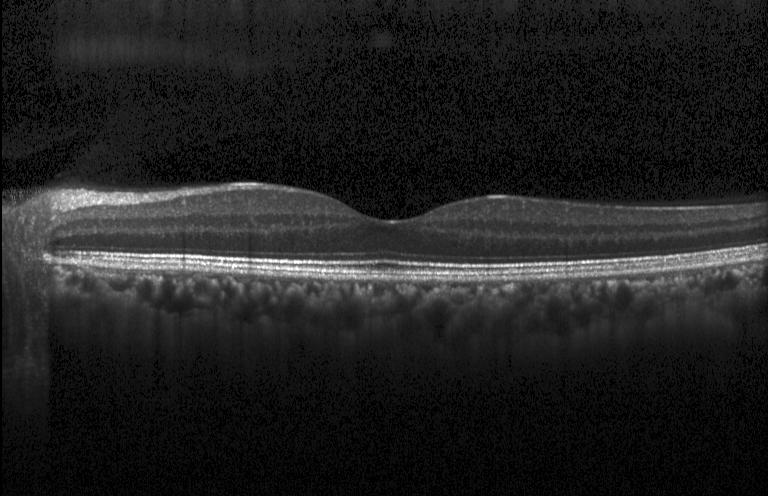

Centered on the fovea, spectral-domain optical coherence tomography, retinal OCT cross-section. OCT finding: no CNV, DME, or drusen.